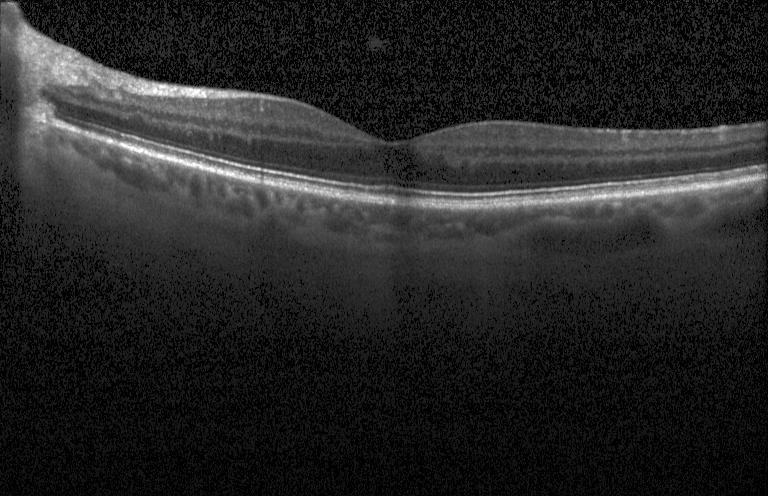

SD-OCT · instrument: Heidelberg Spectralis · centered on the fovea · optical coherence tomography scan.
This B-scan demonstrates no choroidal neovascularization, no diabetic macular edema, and no drusen.